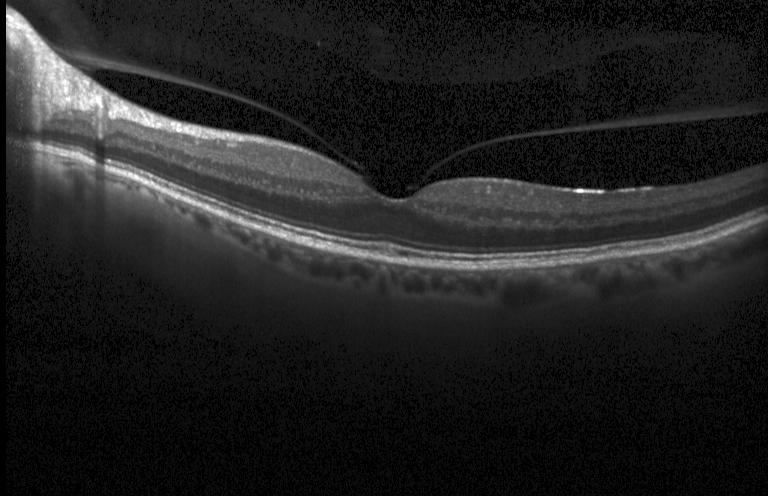
Diagnosis: no choroidal neovascularization, no diabetic macular edema, and no drusen.